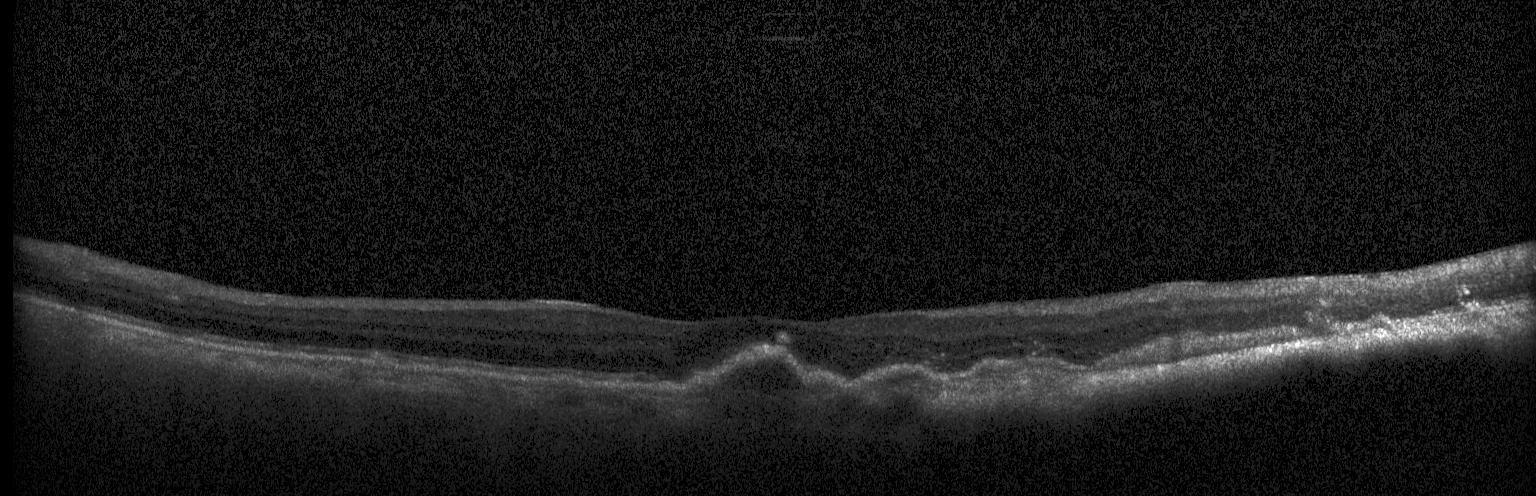
OCT finding: a choroidal neovascular membrane.